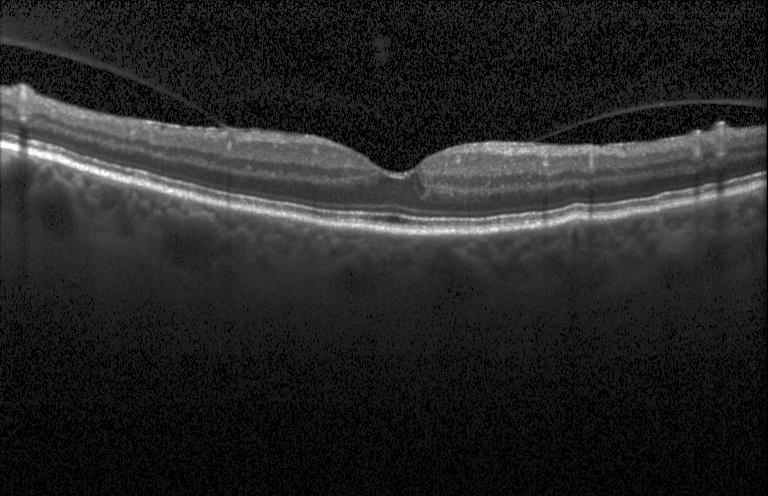

SD-OCT; retinal OCT cross-section; acquired on a Heidelberg Spectralis; through the macula. Diagnosis: neither choroidal neovascularization, diabetic macular edema, nor drusen.